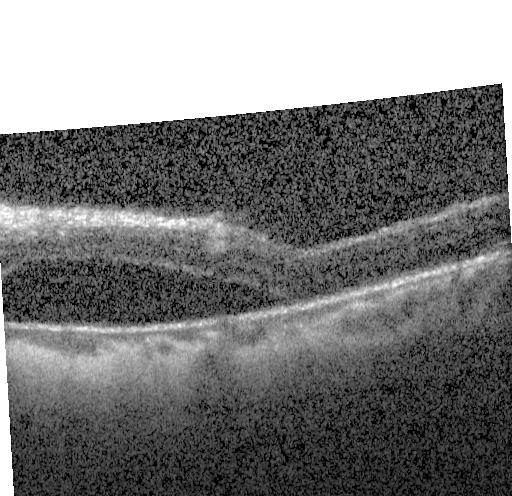
Dx: CNV.